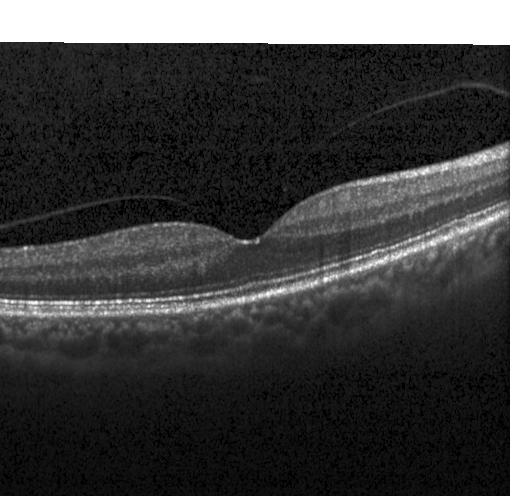

Retinal OCT B-scan; fovea-centered; instrument: Heidelberg Spectralis
Diagnosis: neither choroidal neovascularization, diabetic macular edema, nor drusen.